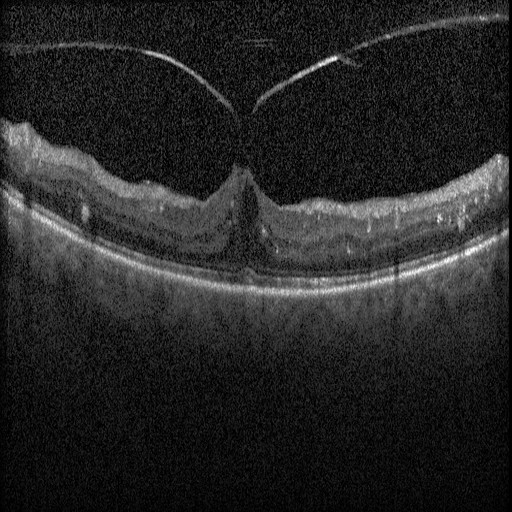

Retinal OCT B-scan, horizontal scan through the fovea
Diagnosis: diabetic macular edema.